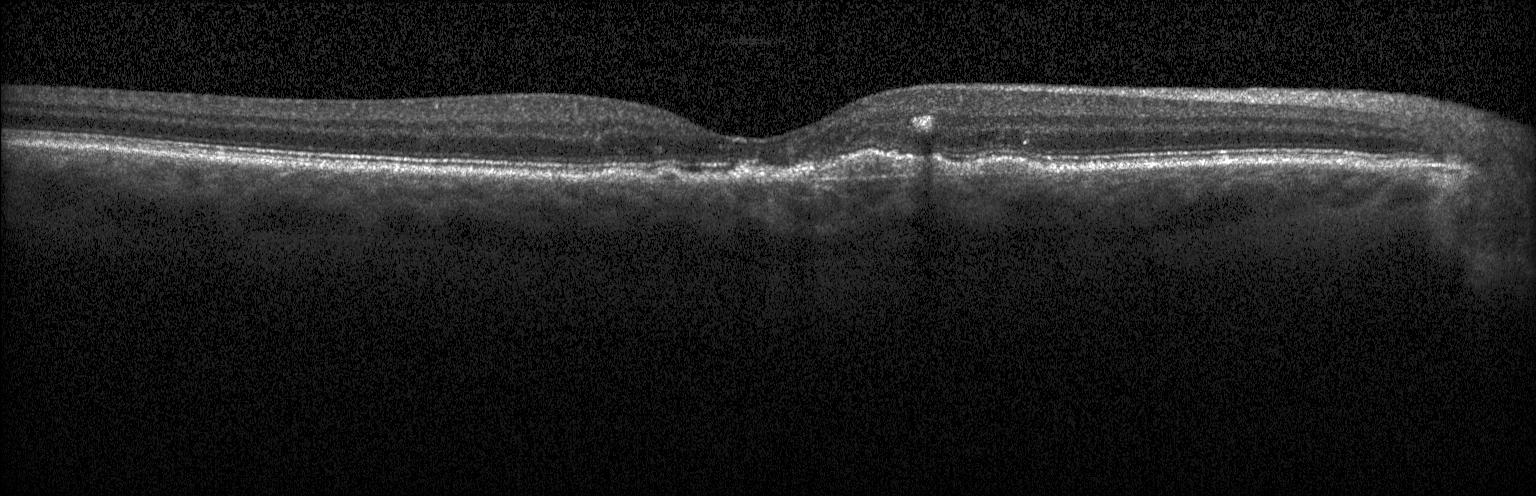

Instrument: Heidelberg Spectralis; SD-OCT; horizontal scan through the fovea; OCT line scan. OCT finding: a choroidal neovascular membrane.